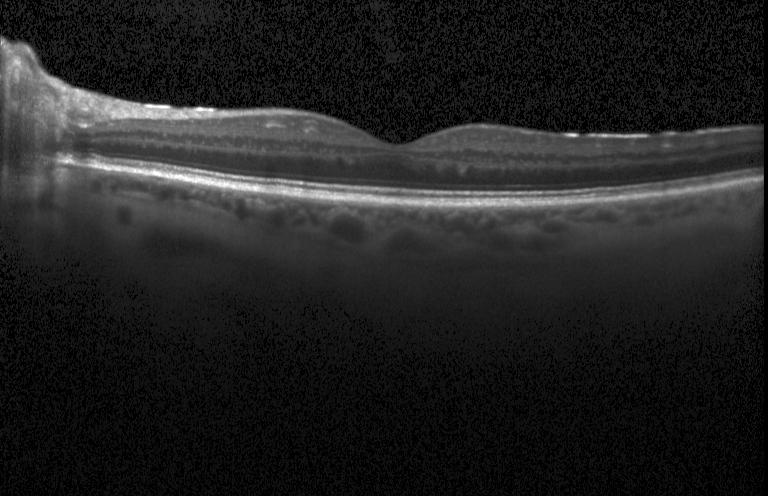

Spectral-domain optical coherence tomography; centered on the fovea; retinal OCT B-scan — No choroidal neovascularization, no diabetic macular edema, and no drusen.